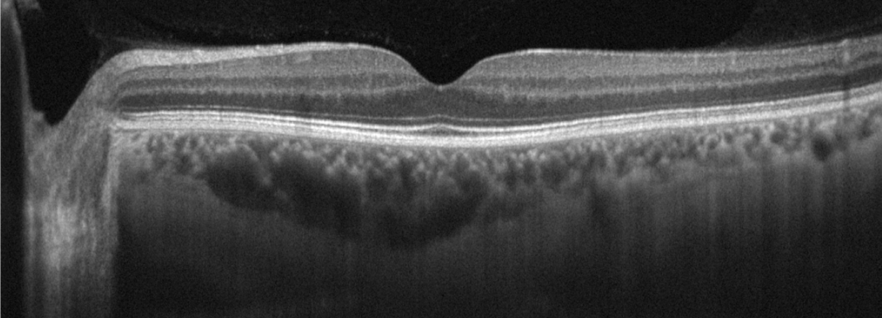

Retinal OCT cross-section. Macular scan.
Absence of AMD, DME, ERM, RAO, RVO, and vitreomacular interface disease.